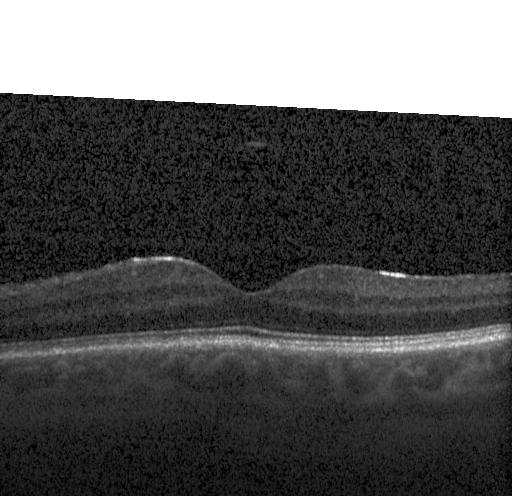 No choroidal neovascularization, diabetic macular edema, or drusen.